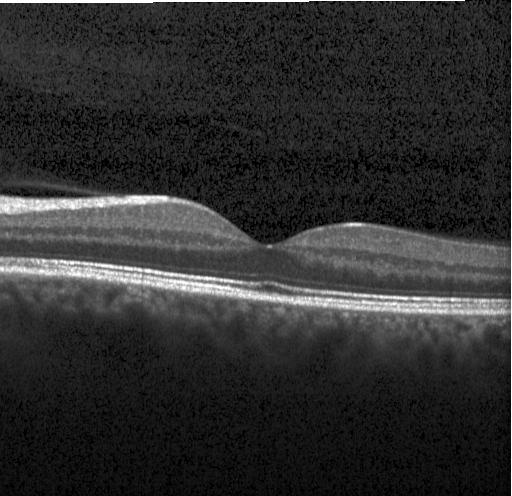
Dx: neither CNV, DME, nor drusen.